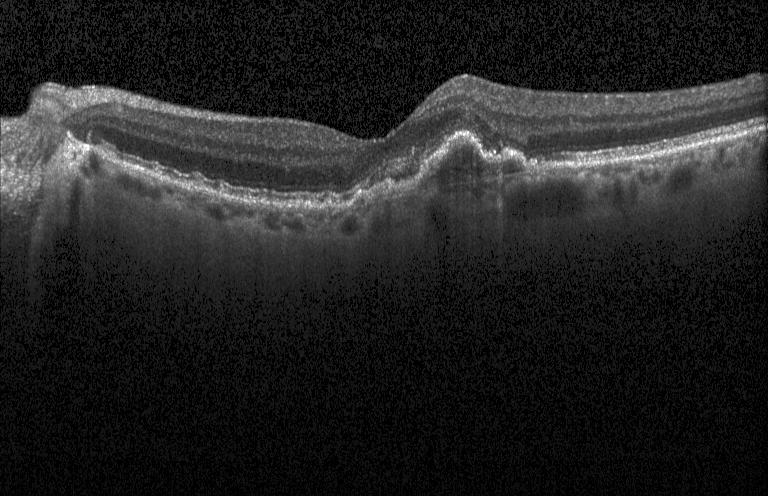

Diagnosis: CNV.